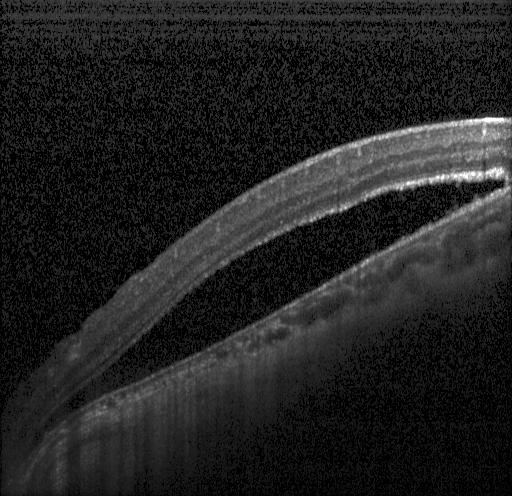

Optical coherence tomography B-scan — The scan shows a choroidal neovascular membrane.